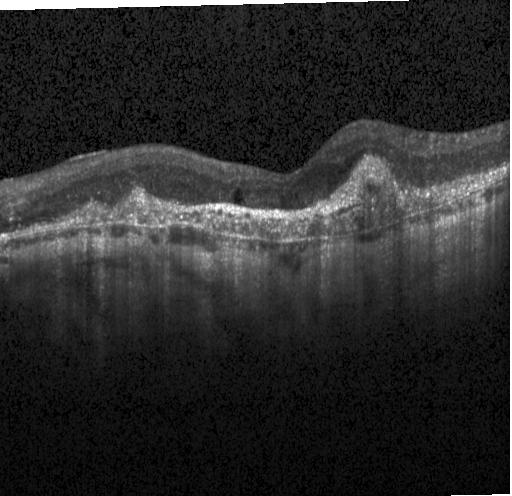
The scan shows CNV.